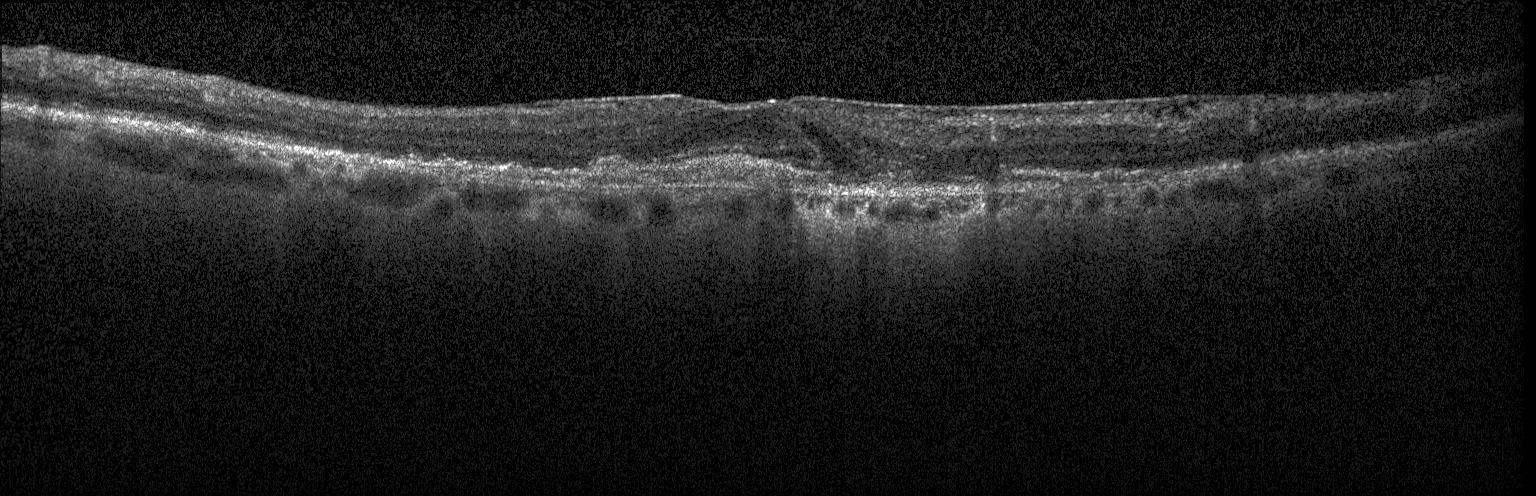 Finding: a choroidal neovascular membrane.